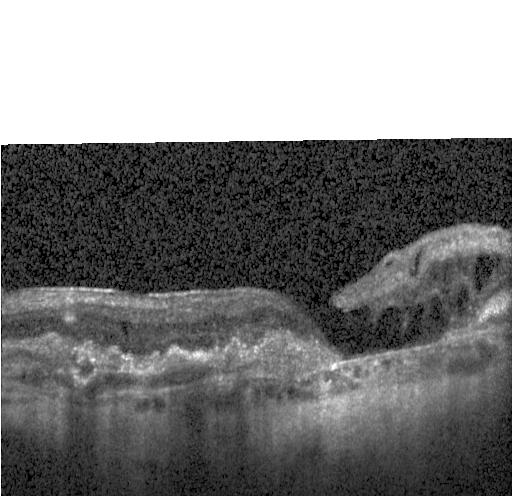

The scan shows CNV.